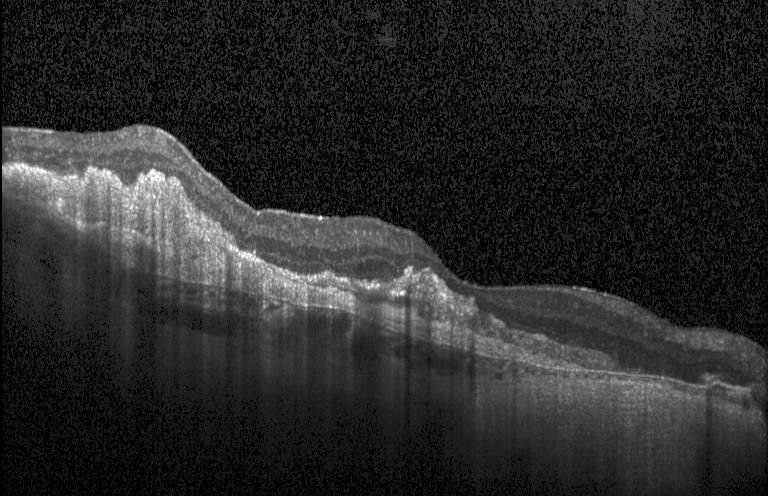
Retinal OCT cross-section, spectral-domain OCT.
This B-scan demonstrates a choroidal neovascular membrane.